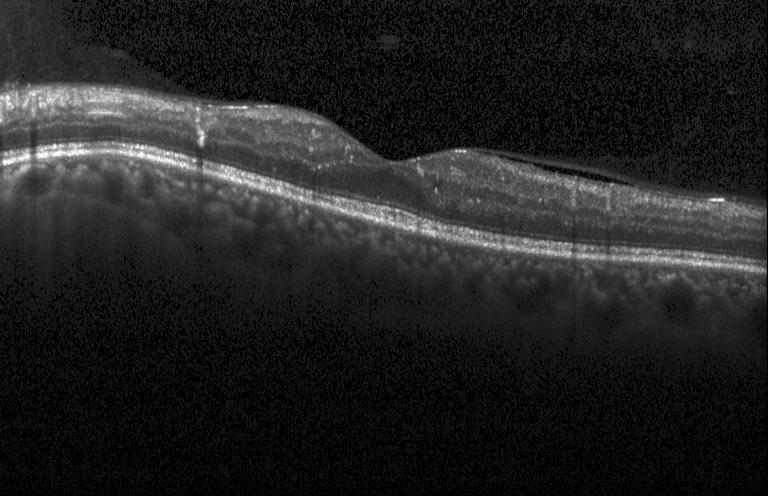 Optical coherence tomography scan · Heidelberg Spectralis OCT system. The scan shows diabetic macular edema (DME).